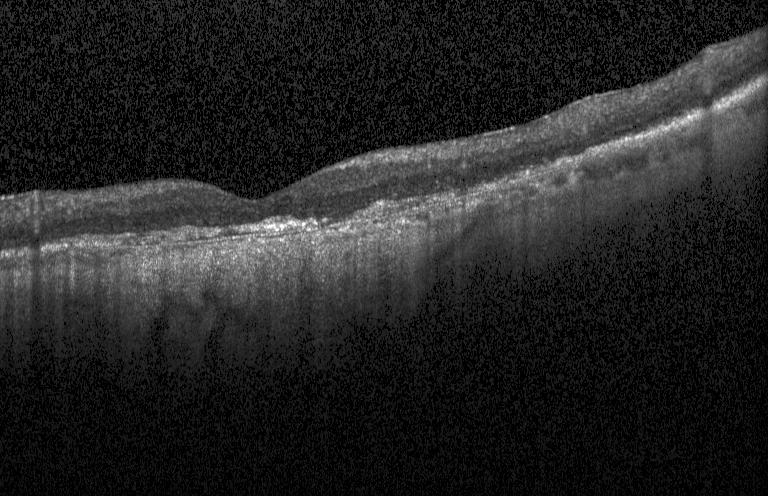

Centered on the fovea, acquired on a Heidelberg Spectralis, retinal OCT B-scan, SD-OCT. Impression: a choroidal neovascular membrane.